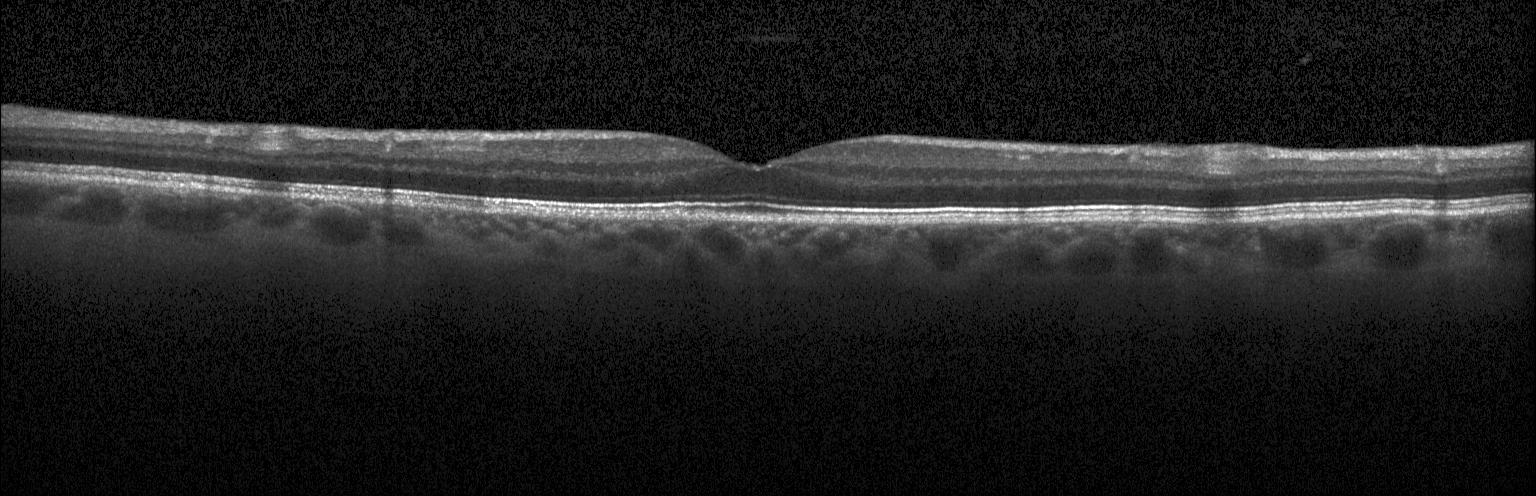

Heidelberg Spectralis. Spectral-domain OCT. OCT line scan.
Impression: no choroidal neovascularization, no diabetic macular edema, and no drusen.